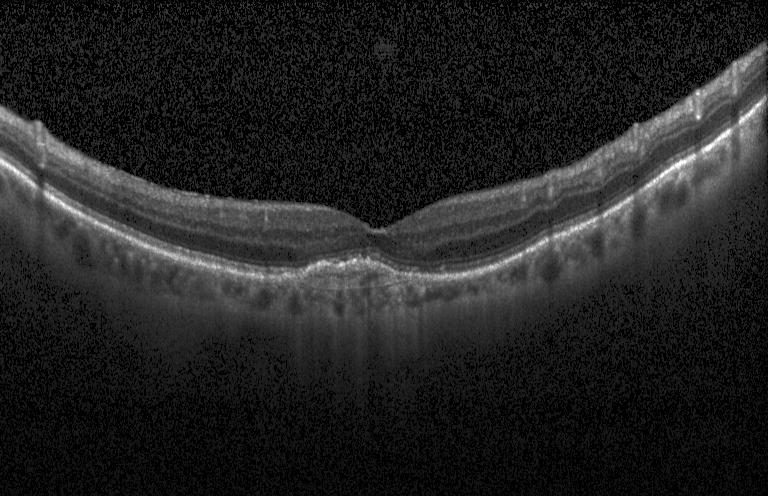
Heidelberg Spectralis OCT system. Centered on the fovea. Retinal OCT cross-section. SD-OCT. Diagnosis: CNV.